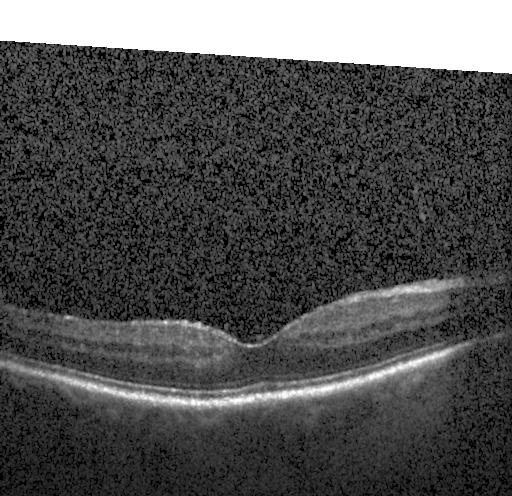
Spectral-domain optical coherence tomography · horizontal scan through the fovea · optical coherence tomography B-scan · instrument: Heidelberg Spectralis
The scan shows no CNV, DME, or drusen.